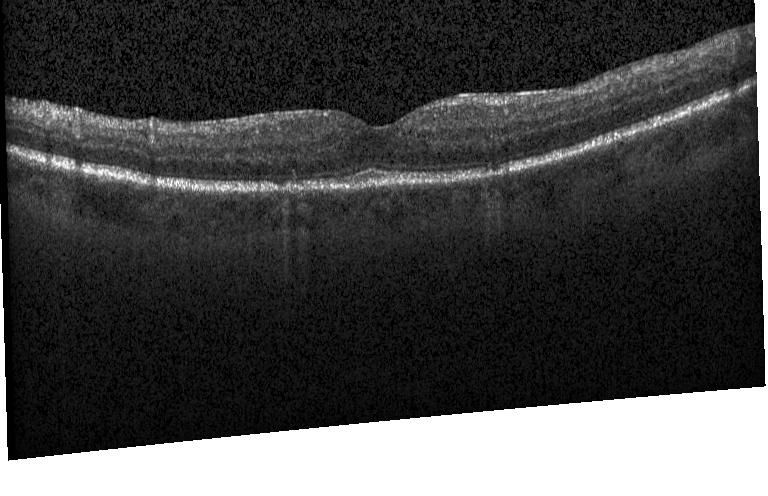 OCT line scan, fovea-centered. Finding: DME.